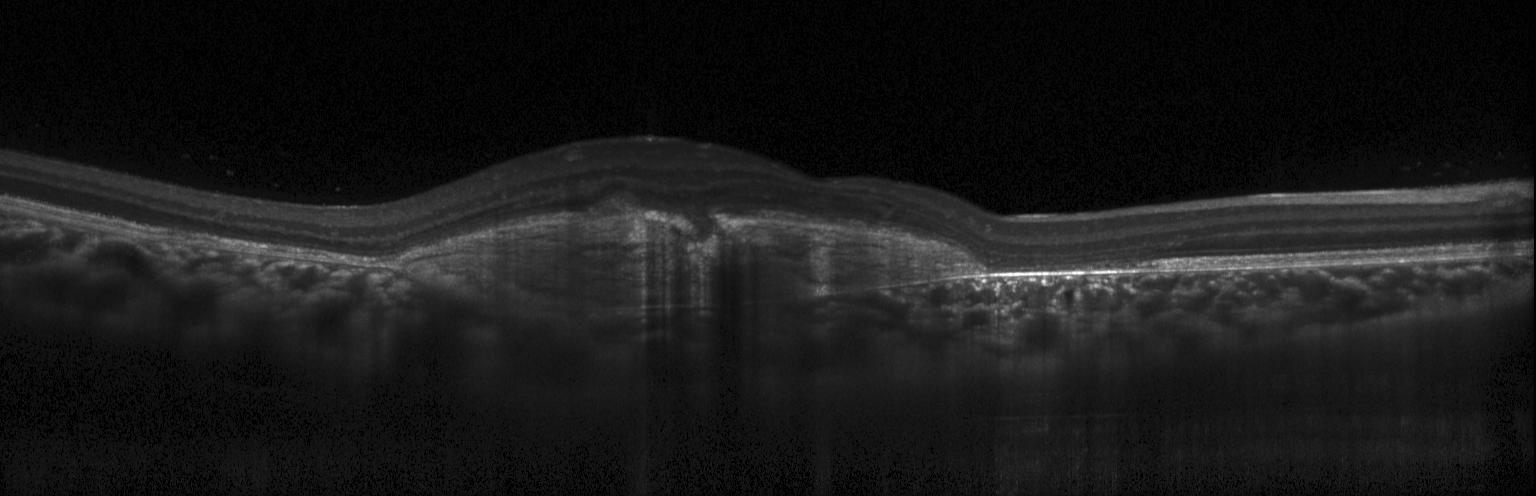
Retinal OCT cross-section — Diagnosis: choroidal neovascularization (CNV).